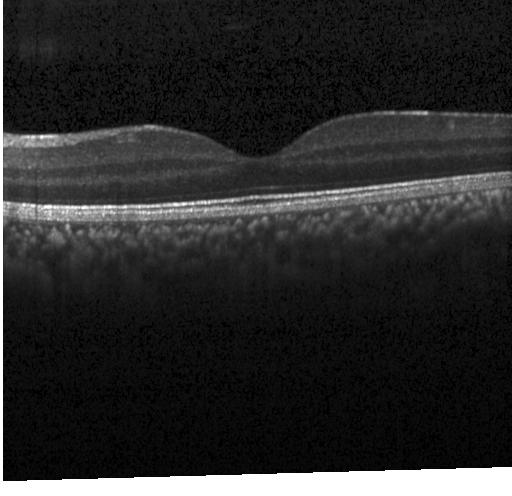
OCT finding: no choroidal neovascularization, no diabetic macular edema, and no drusen.